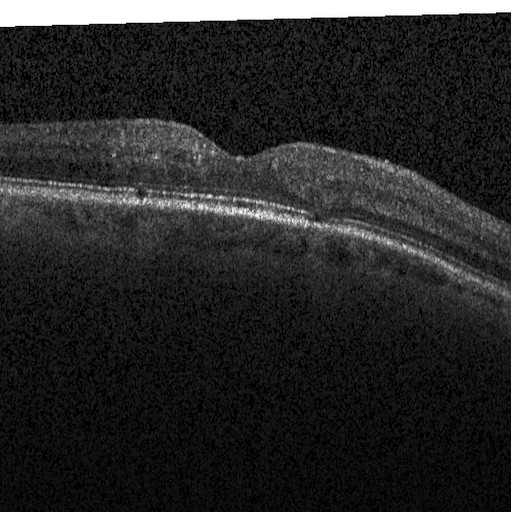

Retinal OCT B-scan. Assessment: diabetic macular edema.